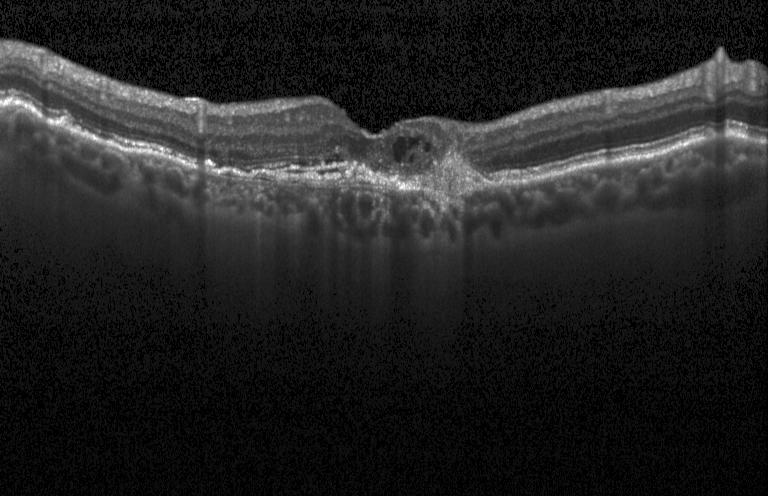 OCT B-scan showing choroidal neovascularization (CNV).